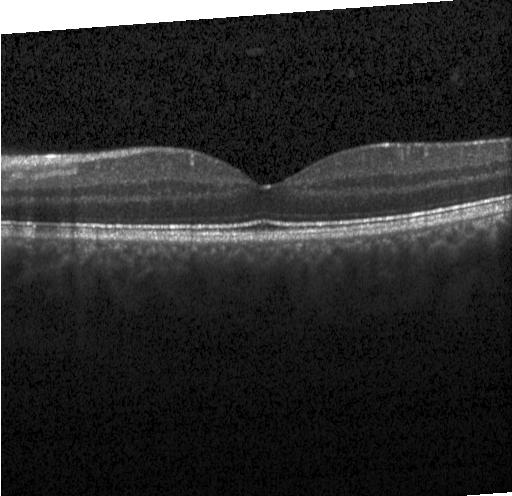

Retinal OCT B-scan · Heidelberg Spectralis OCT system · fovea-centered. Diagnosis: no choroidal neovascularization, diabetic macular edema, or drusen.